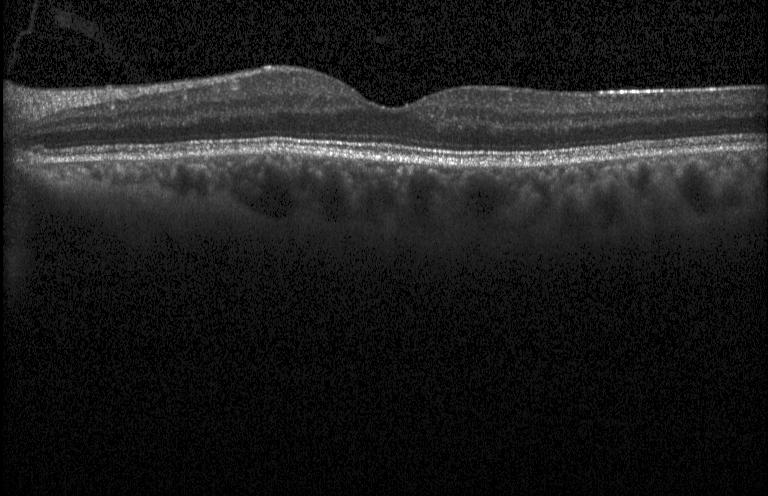
Optical coherence tomography B-scan. Finding: no evidence of choroidal neovascularization, diabetic macular edema, or drusen.